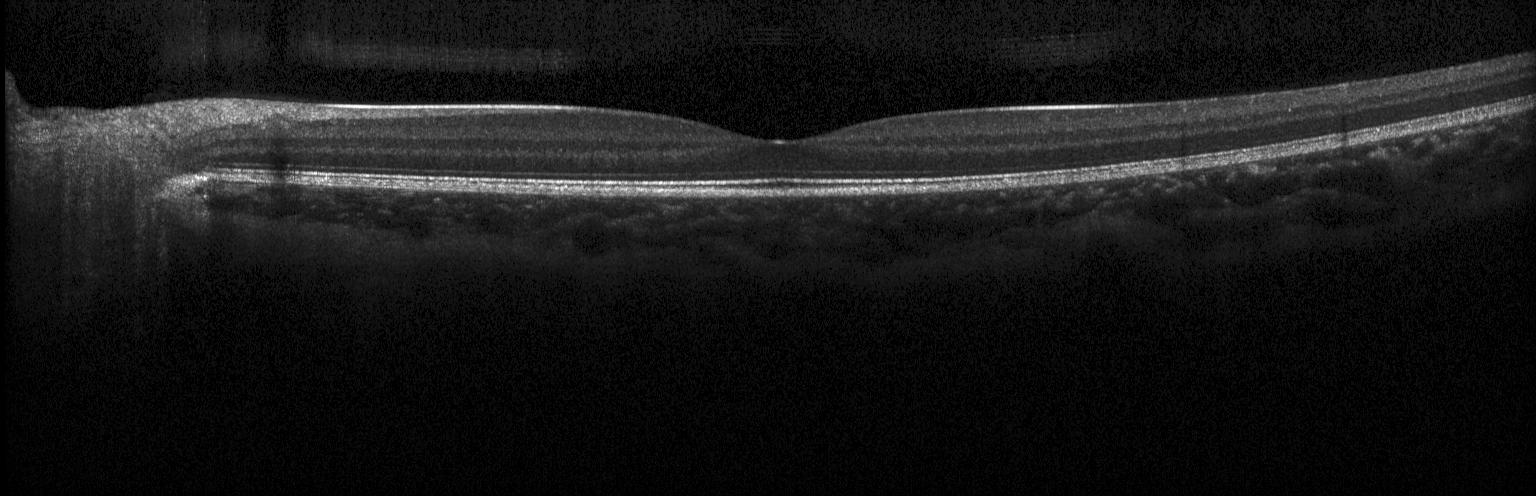

Heidelberg Spectralis OCT system. Retinal OCT B-scan
Finding: no evidence of choroidal neovascularization, diabetic macular edema, or drusen.